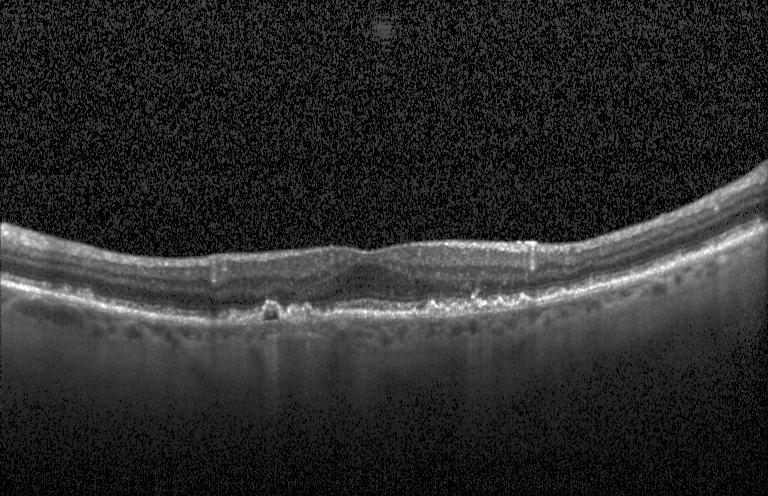

OCT finding: multiple drusen.